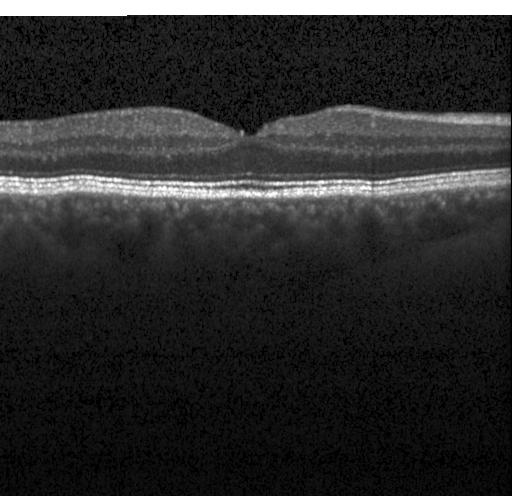

Diagnosis: neither choroidal neovascularization, diabetic macular edema, nor drusen.